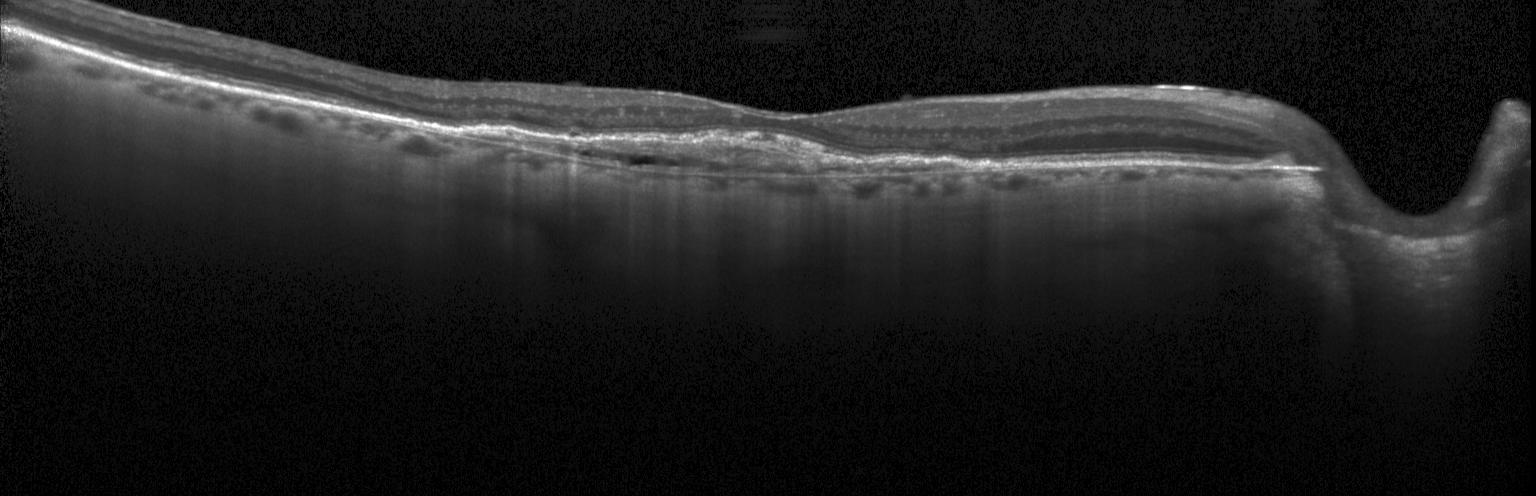 This B-scan demonstrates a choroidal neovascular membrane.